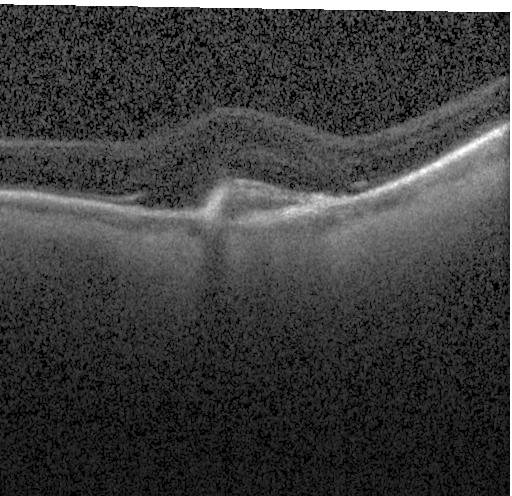
Dx: a choroidal neovascular membrane.